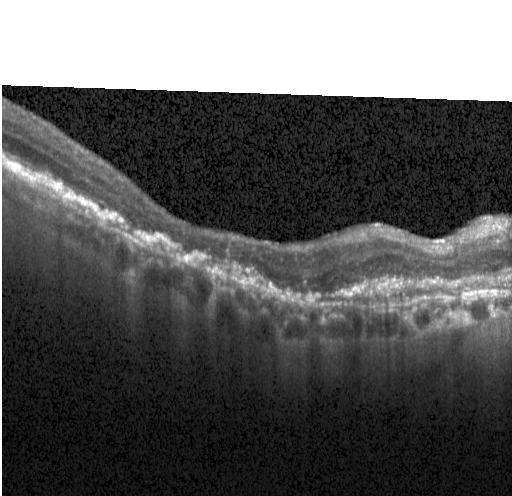
Retinal OCT B-scan
Finding: a choroidal neovascular membrane.